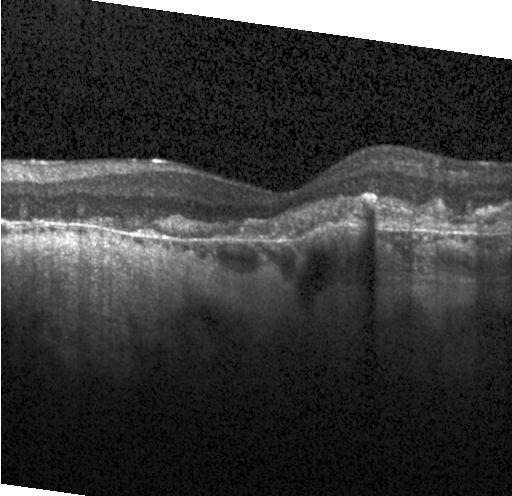

OCT B-scan showing a choroidal neovascular membrane.